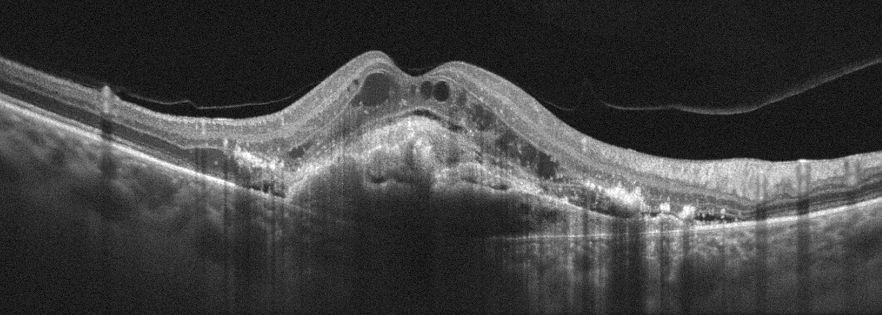
Retinal OCT cross-section showing age-related macular degeneration.